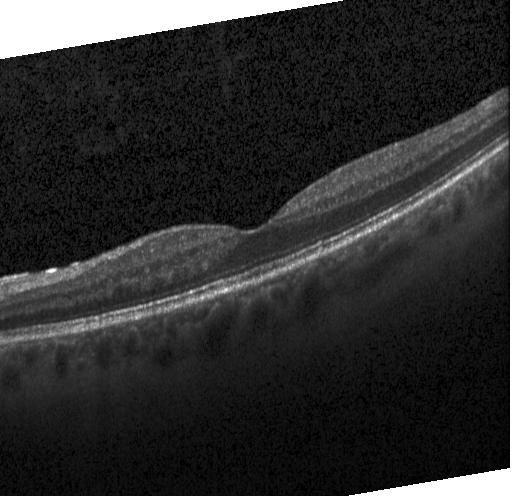 OCT B-scan showing neither CNV, DME, nor drusen.